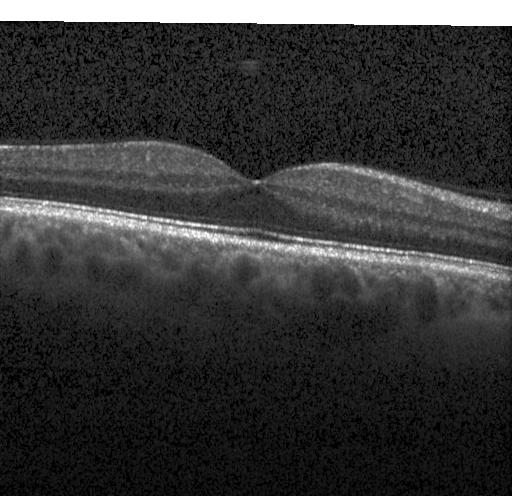 SD-OCT · acquired on a Heidelberg Spectralis · OCT B-scan — Diagnosis: no evidence of choroidal neovascularization, diabetic macular edema, or drusen.